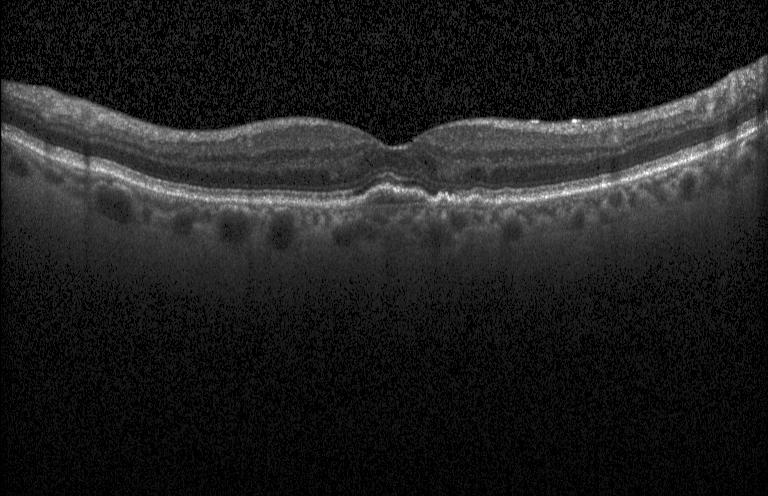
Acquired on a Heidelberg Spectralis, SD-OCT, through the macula, optical coherence tomography scan.
Impression: CNV.